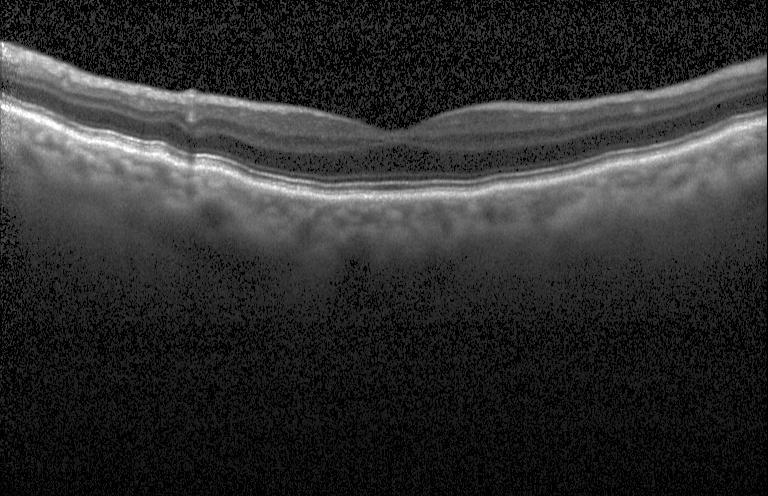
Impression: no choroidal neovascularization, diabetic macular edema, or drusen.